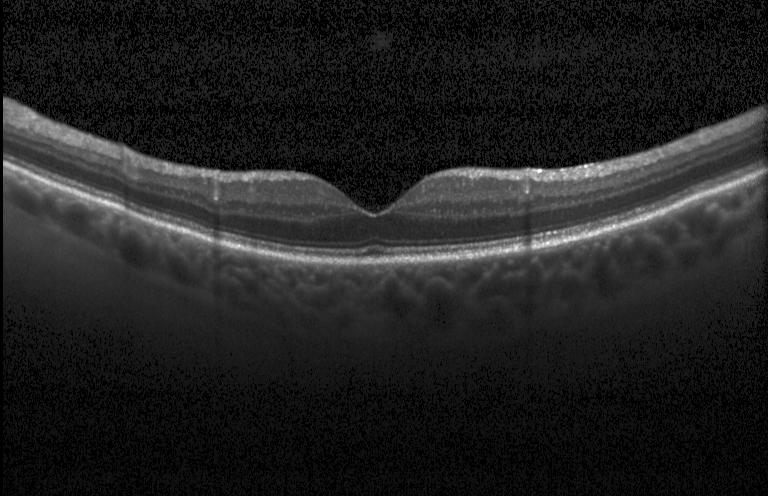

Finding: no CNV, DME, or drusen.